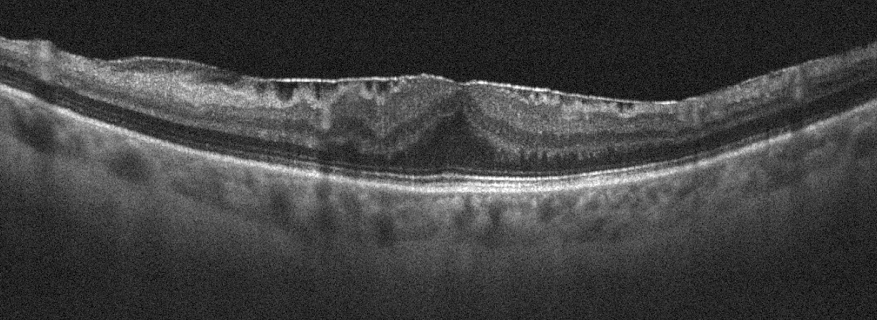
Optical coherence tomography B-scan; macular scan; Optovue Avanti RTVue XR.
Finding: epiretinal membrane (ERM).